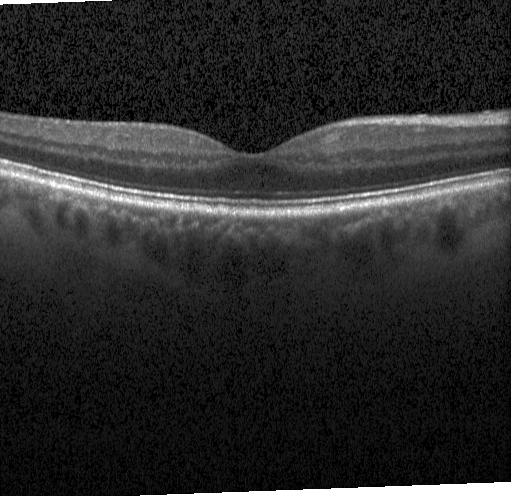 Instrument: Heidelberg Spectralis. Optical coherence tomography scan — Impression: no evidence of choroidal neovascularization, diabetic macular edema, or drusen.